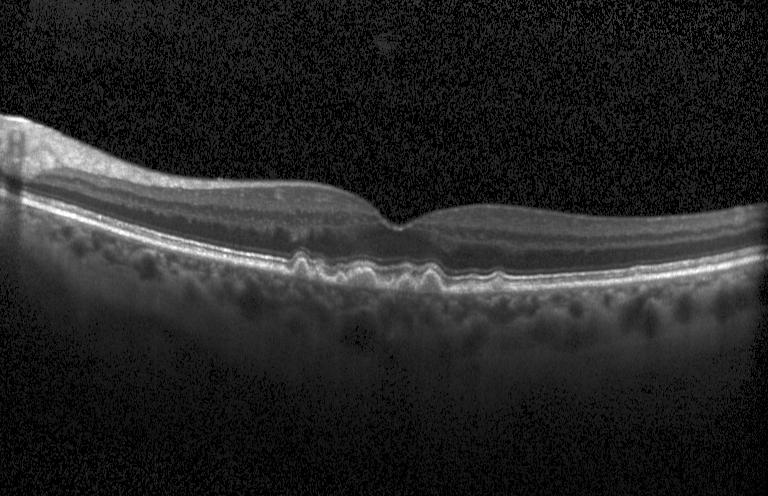

Retinal OCT cross-section; through the macula — Diagnosis: sub-RPE drusenoid deposits.